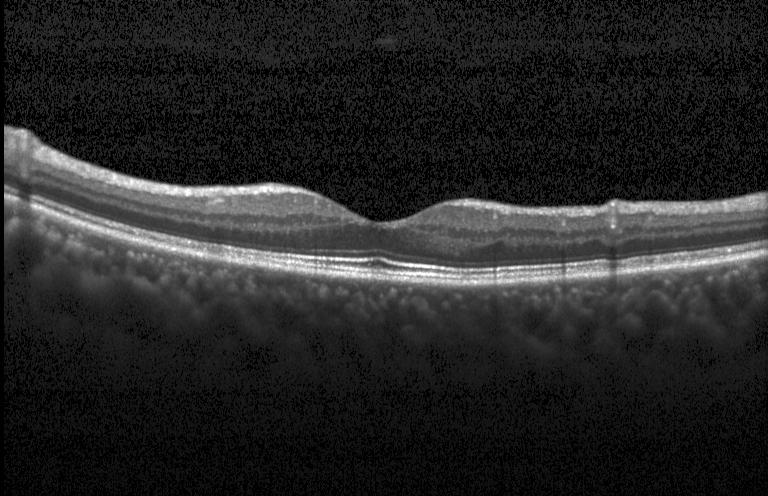 Optical coherence tomography scan. Diagnosis: no CNV, no DME, and no drusen.